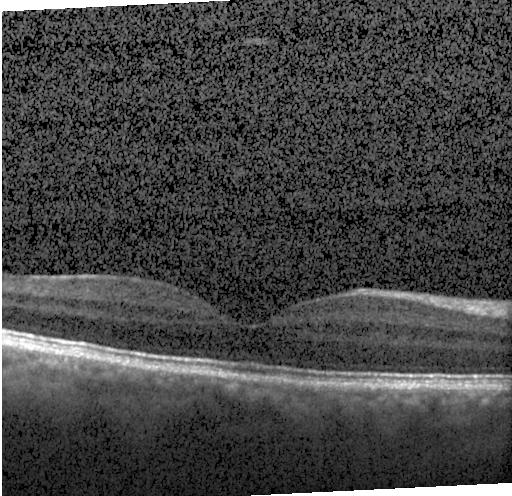 The scan shows no evidence of choroidal neovascularization, diabetic macular edema, or drusen.